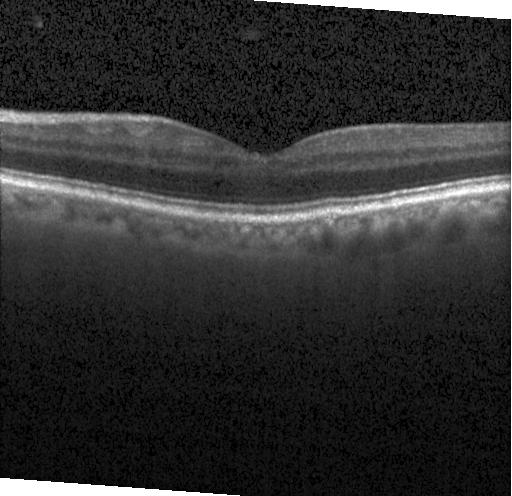 SD-OCT · optical coherence tomography scan. Macular OCT: no choroidal neovascularization, diabetic macular edema, or drusen.